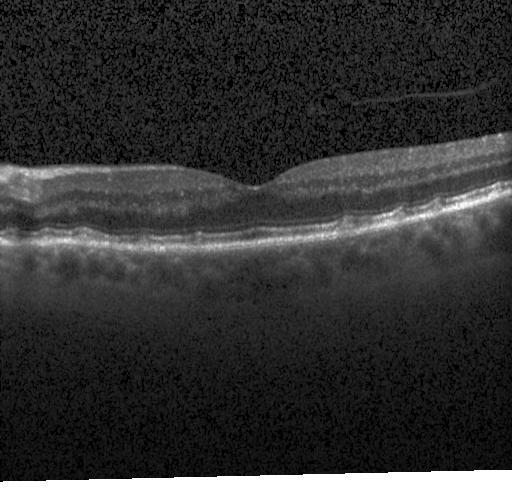 OCT B-scan showing drusen.